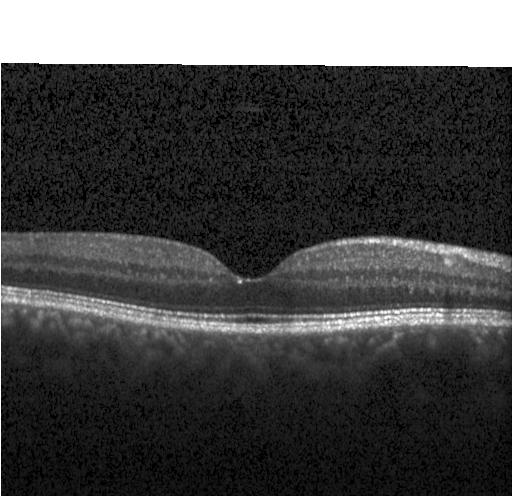 Centered on the fovea. Spectral-domain optical coherence tomography. Heidelberg Spectralis. Optical coherence tomography scan — Assessment: neither CNV, DME, nor drusen.